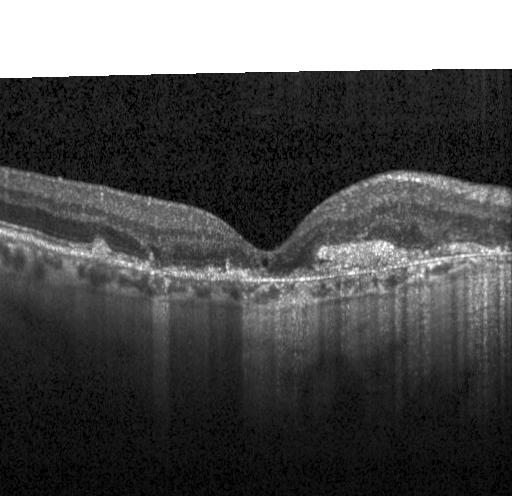 Optical coherence tomography B-scan; centered on the fovea; SD-OCT
Assessment: choroidal neovascularization.